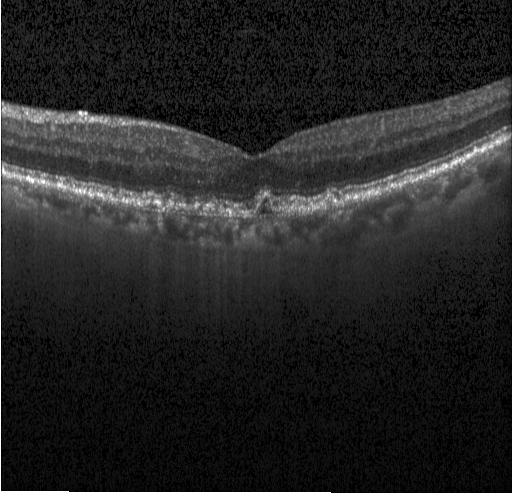

Instrument: Heidelberg Spectralis. Through the macula. Optical coherence tomography scan. SD-OCT.
This B-scan demonstrates a choroidal neovascular membrane.